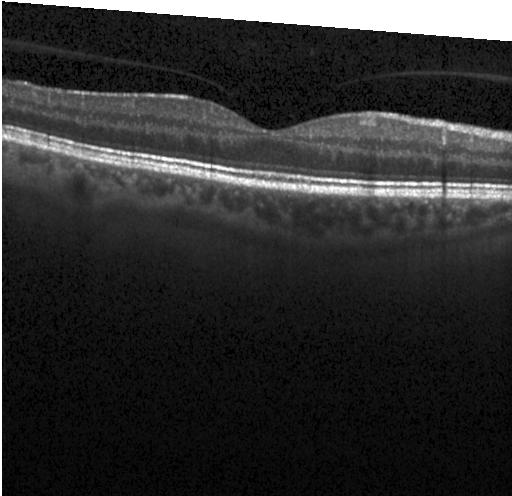

Diagnosis: no choroidal neovascularization, diabetic macular edema, or drusen.